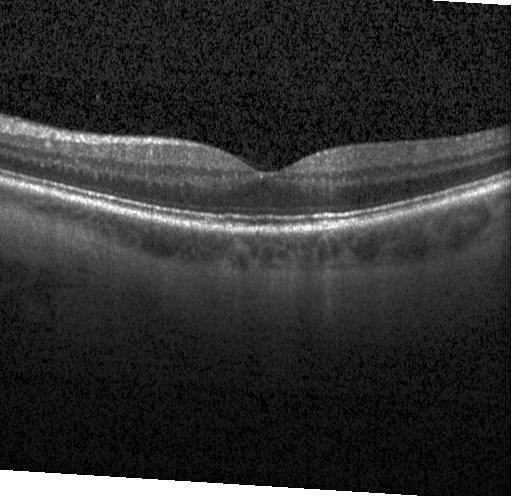

Optical coherence tomography B-scan — Finding: neither choroidal neovascularization, diabetic macular edema, nor drusen.